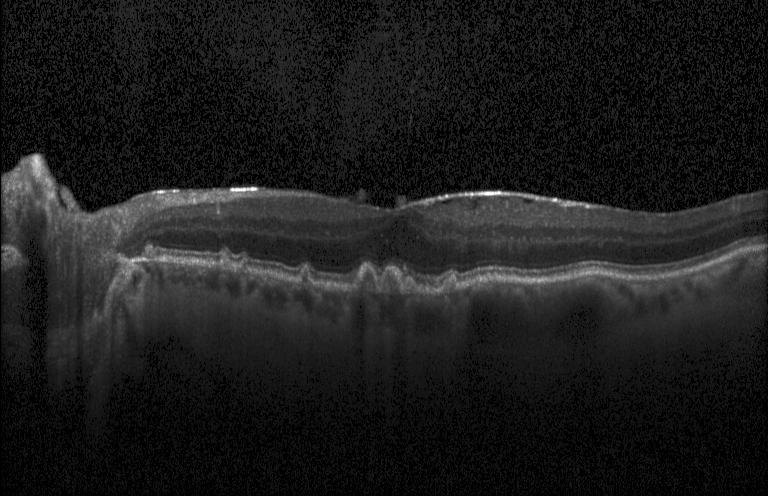 OCT B-scan. OCT finding: drusen.